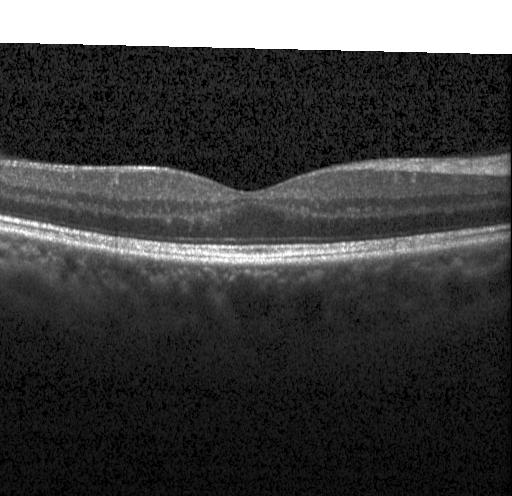
Macular scan. Optical coherence tomography B-scan. Spectral-domain OCT — No evidence of choroidal neovascularization, diabetic macular edema, or drusen.